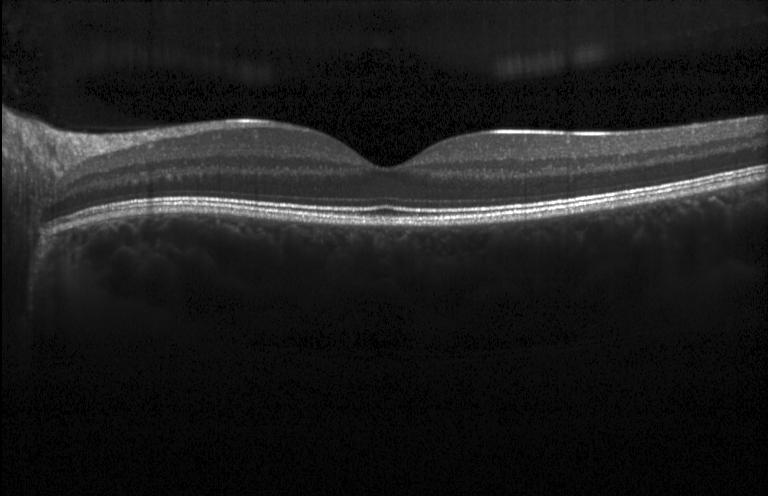

Assessment: neither choroidal neovascularization, diabetic macular edema, nor drusen.